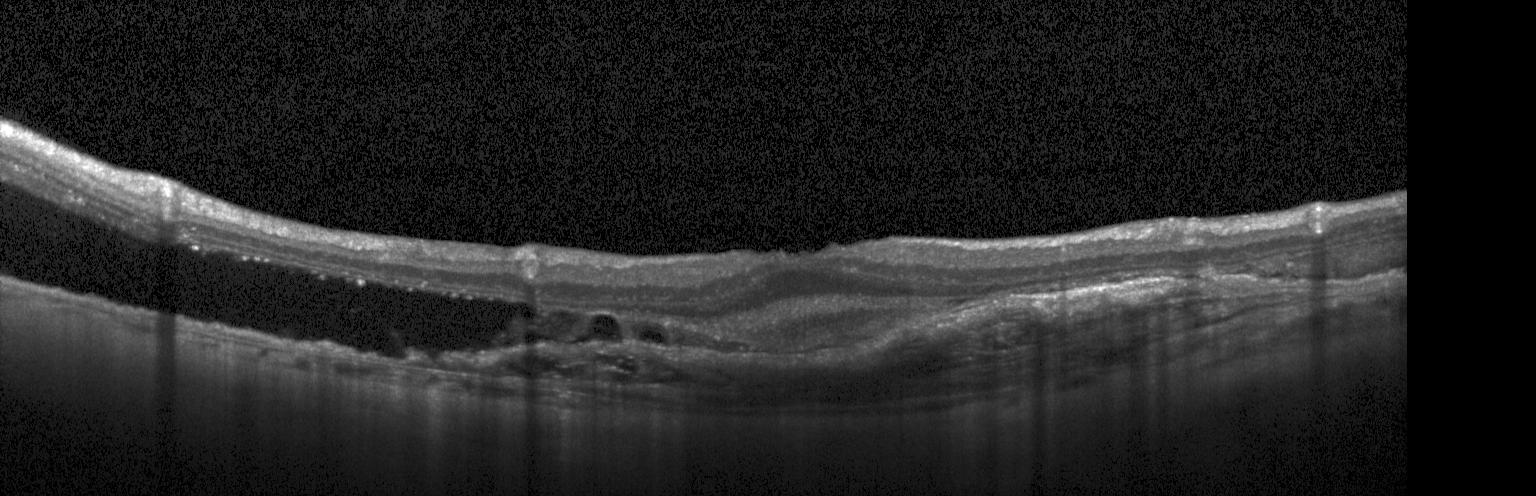
CNV.